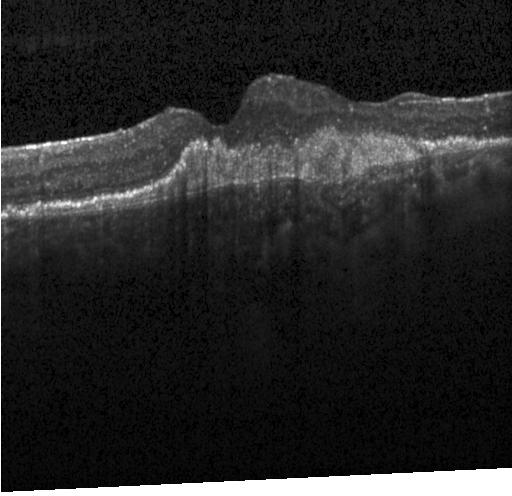
OCT B-scan
Dx: choroidal neovascularization.